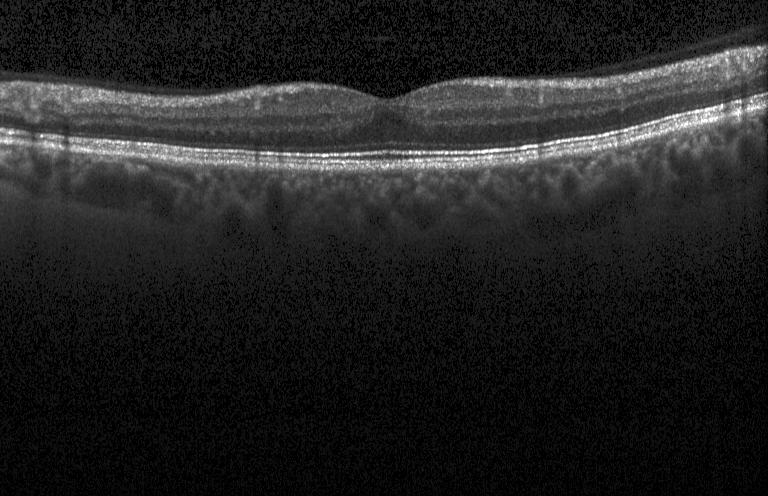

Acquired on a Heidelberg Spectralis, fovea-centered, OCT B-scan
The scan shows no choroidal neovascularization, no diabetic macular edema, and no drusen.